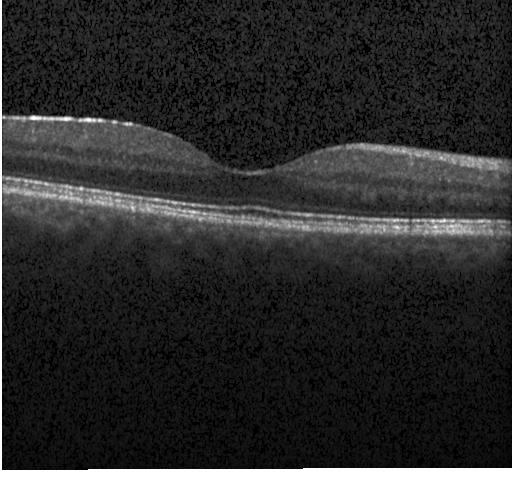 Optical coherence tomography scan. This B-scan demonstrates neither choroidal neovascularization, diabetic macular edema, nor drusen.